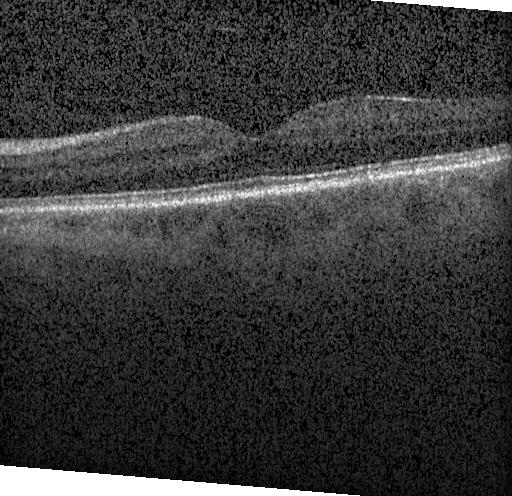

OCT finding: no evidence of choroidal neovascularization, diabetic macular edema, or drusen.